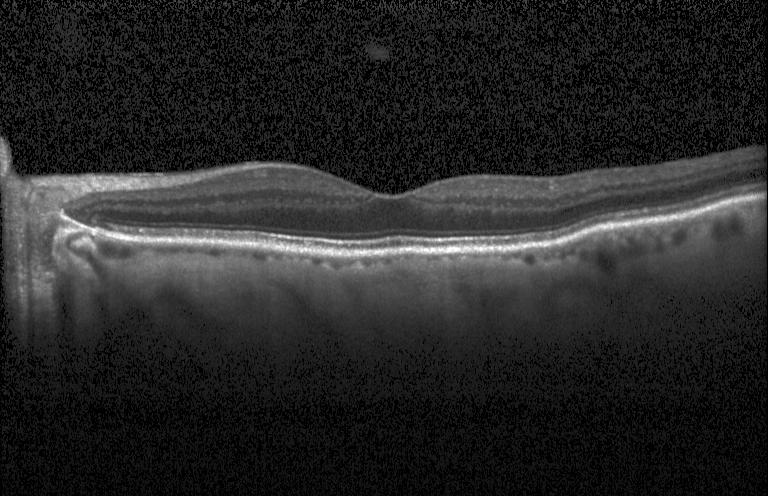
OCT line scan — Finding: no CNV, no DME, and no drusen.